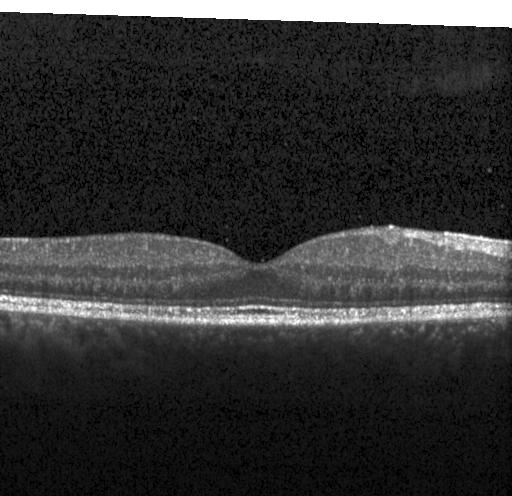
OCT line scan · SD-OCT — Dx: no choroidal neovascularization, diabetic macular edema, or drusen.